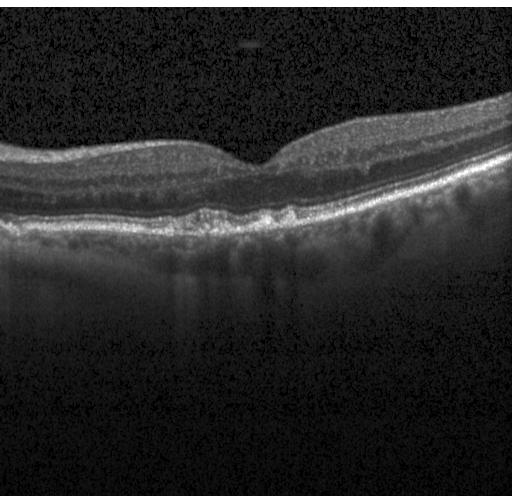
Macular OCT demonstrating sub-RPE drusenoid deposits.